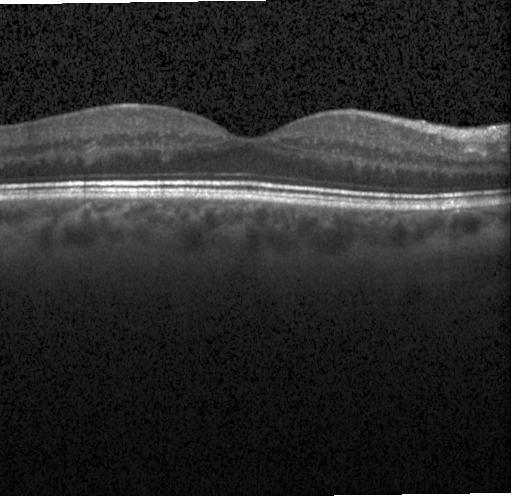 Retinal OCT cross-section.
No CNV, no DME, and no drusen.